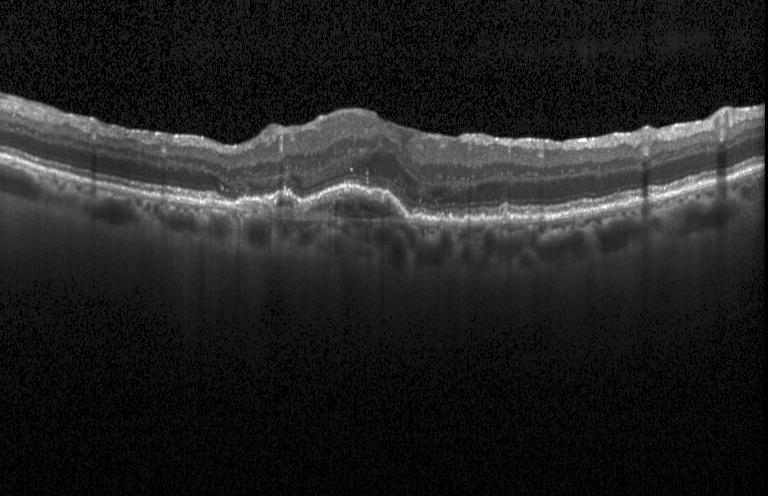

Finding: choroidal neovascularization.